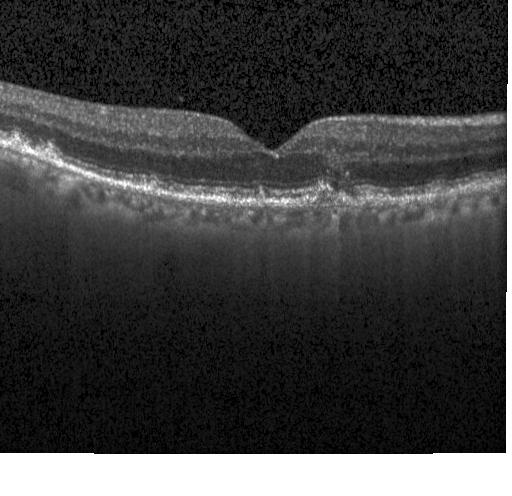 Finding: sub-RPE drusenoid deposits.